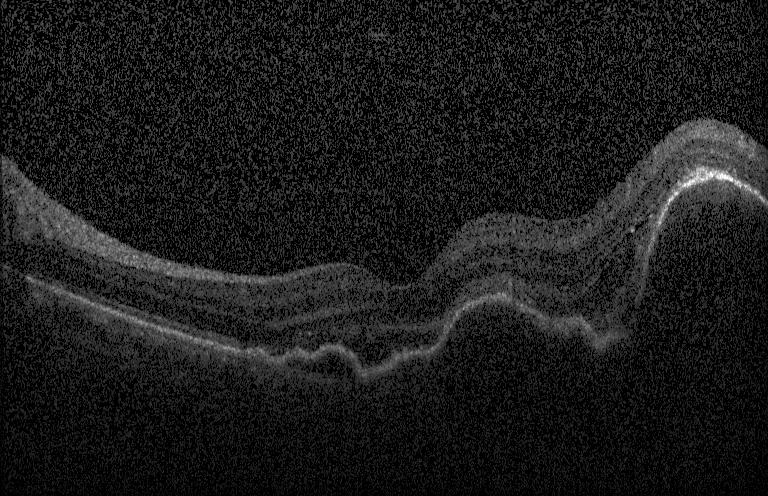
Diagnosis: CNV.